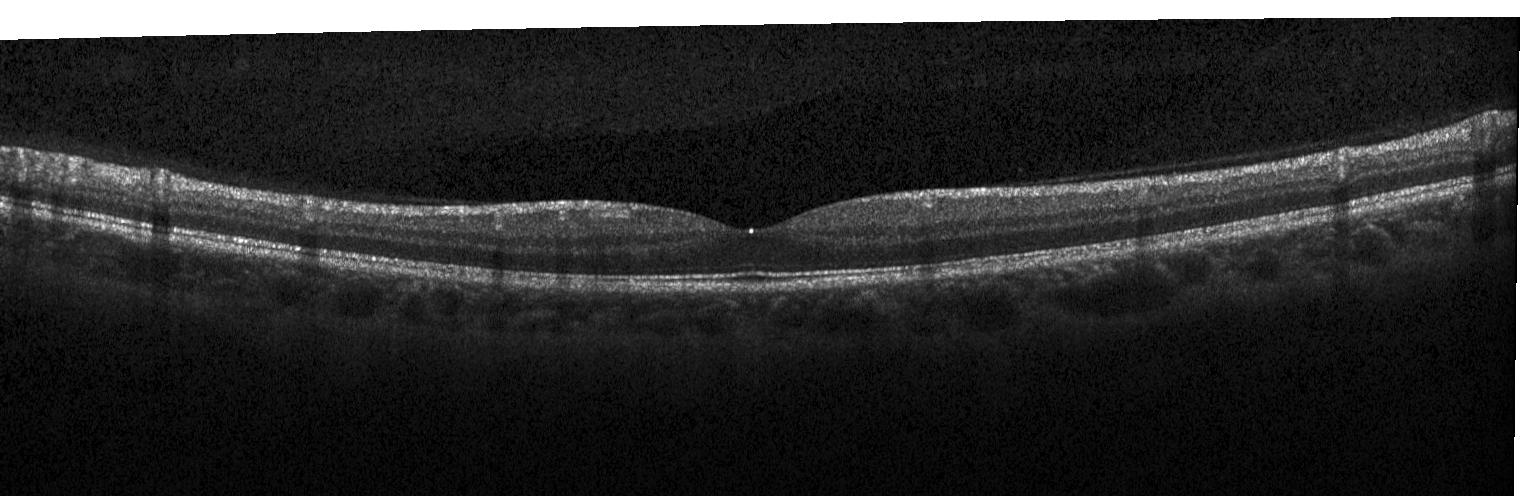
Optical coherence tomography scan; through the macula; Heidelberg Spectralis; spectral-domain optical coherence tomography — Finding: no evidence of choroidal neovascularization, diabetic macular edema, or drusen.